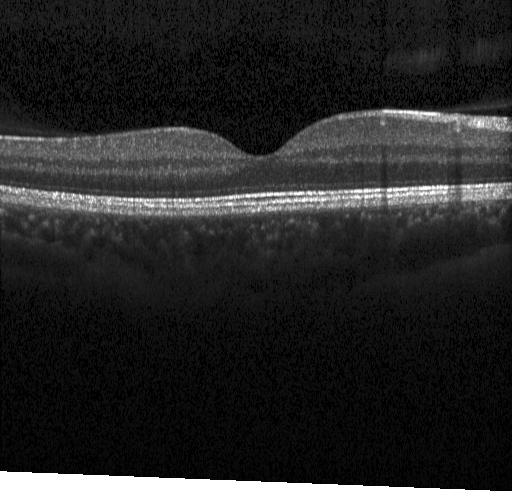

Optical coherence tomography B-scan · Heidelberg Spectralis — Impression: no evidence of choroidal neovascularization, diabetic macular edema, or drusen.